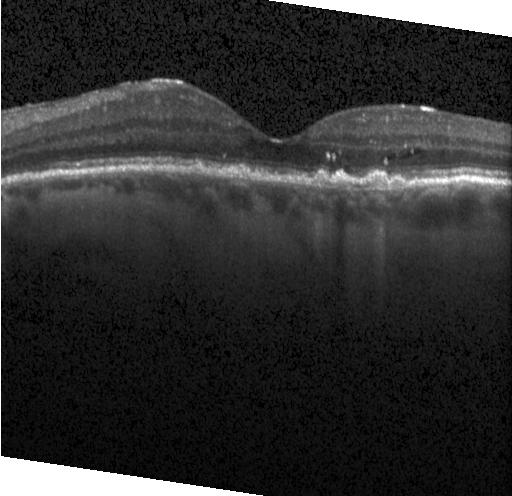

Spectral-domain OCT. Optical coherence tomography B-scan — OCT finding: sub-RPE drusenoid deposits.